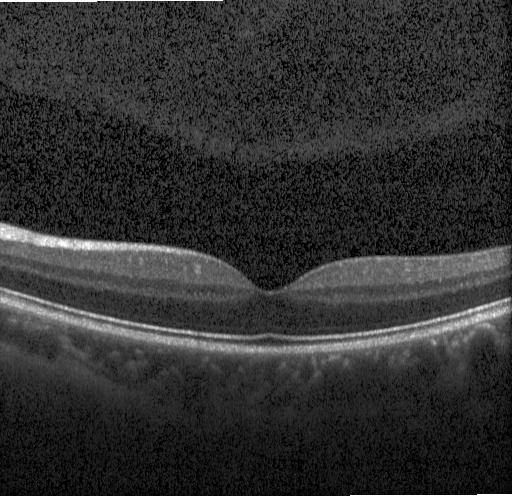
Retinal OCT B-scan. Finding: no evidence of choroidal neovascularization, diabetic macular edema, or drusen.